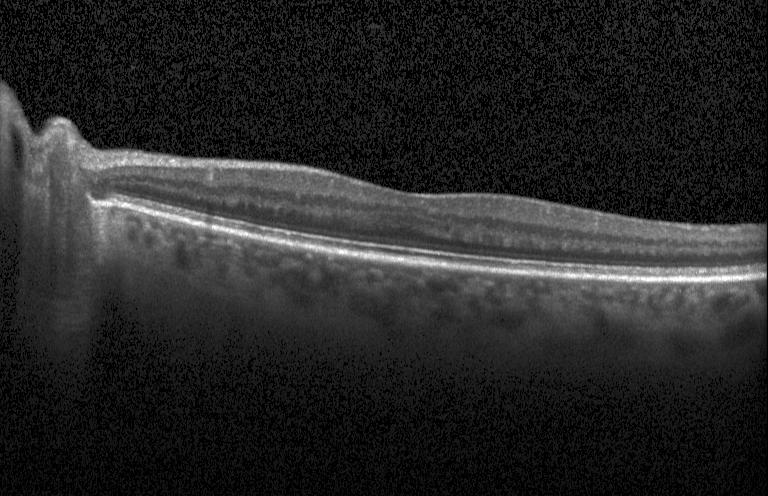 OCT finding: neither choroidal neovascularization, diabetic macular edema, nor drusen.